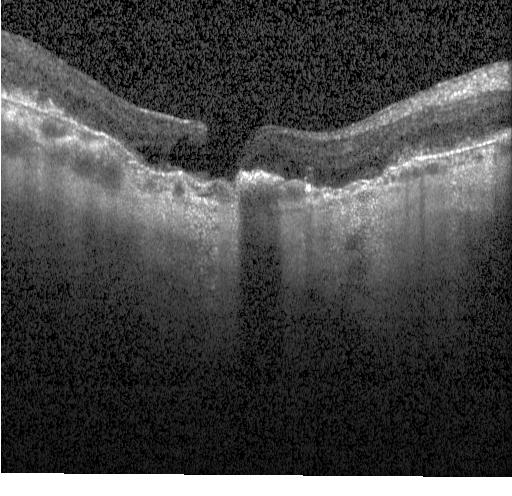 Retinal OCT B-scan — This B-scan demonstrates a choroidal neovascular membrane.